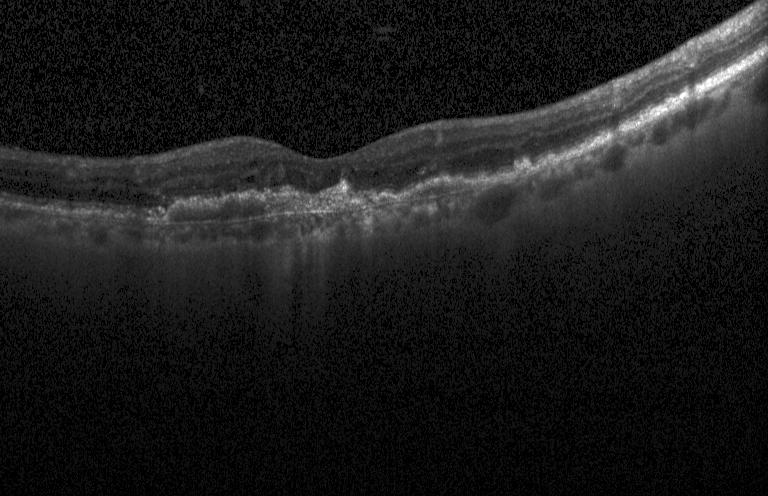 Acquired on a Heidelberg Spectralis, horizontal scan through the fovea, optical coherence tomography scan.
Macular OCT: a choroidal neovascular membrane.